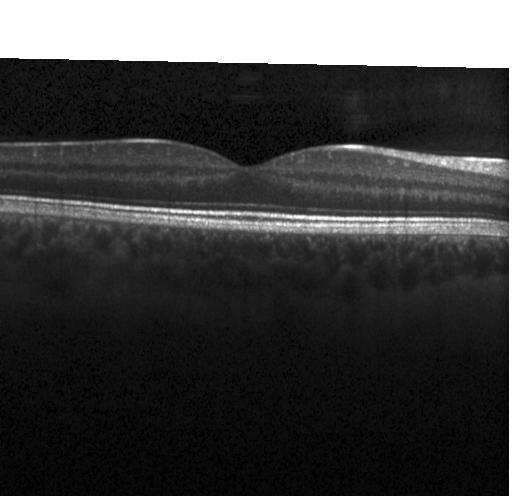
OCT line scan. SD-OCT
Impression: no choroidal neovascularization, diabetic macular edema, or drusen.